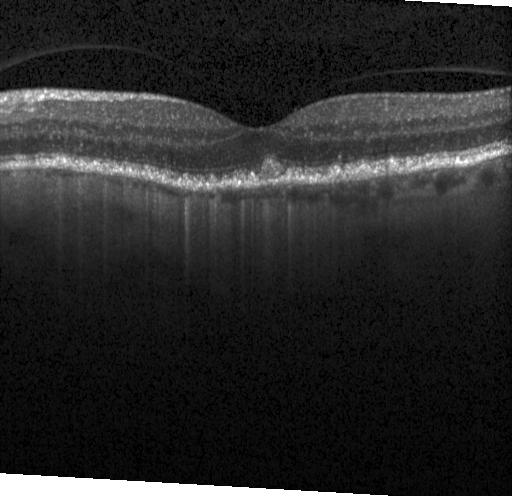
Heidelberg Spectralis OCT system · horizontal scan through the fovea · optical coherence tomography B-scan · spectral-domain OCT
This B-scan demonstrates multiple drusen.